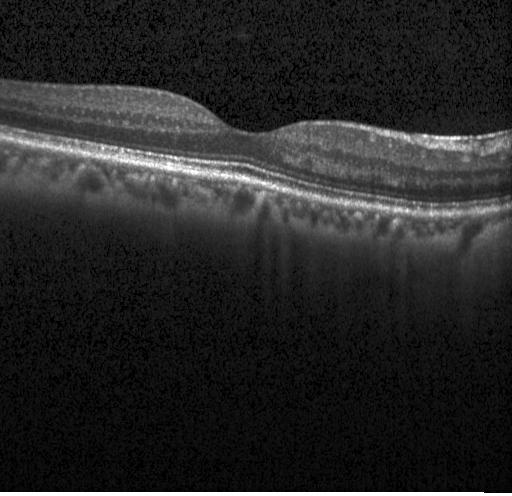
OCT B-scan; horizontal scan through the fovea — The scan shows no choroidal neovascularization, no diabetic macular edema, and no drusen.